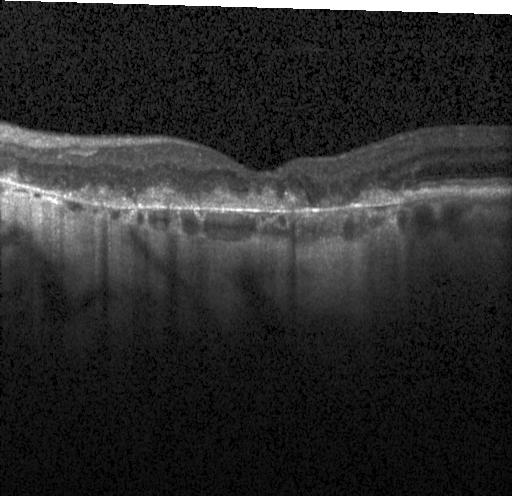

Retinal OCT B-scan — This B-scan demonstrates a choroidal neovascular membrane.